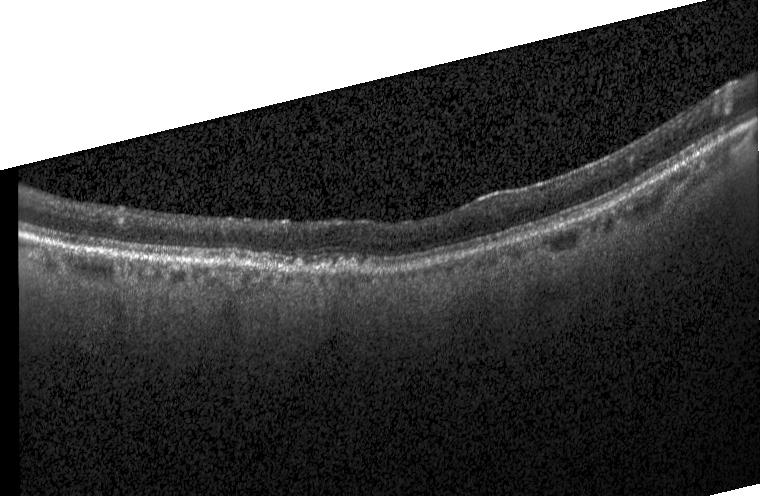
Spectral-domain OCT B-scan: sub-RPE drusenoid deposits.